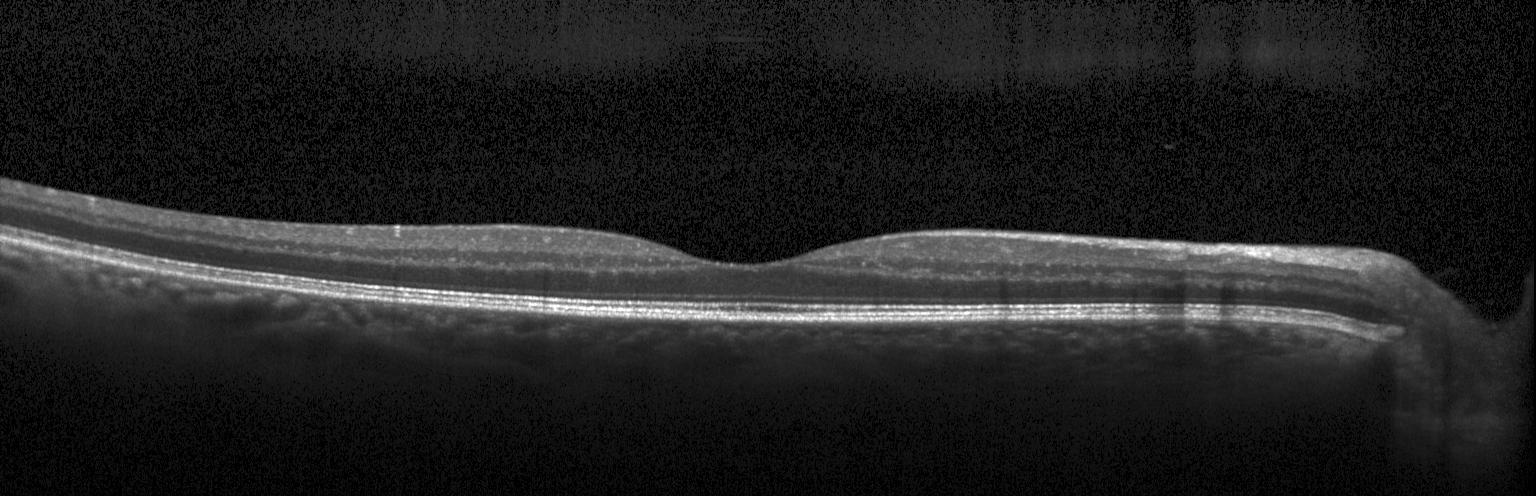
Retinal OCT cross-section · spectral-domain optical coherence tomography · through the macula · Heidelberg Spectralis OCT system.
No choroidal neovascularization, no diabetic macular edema, and no drusen.